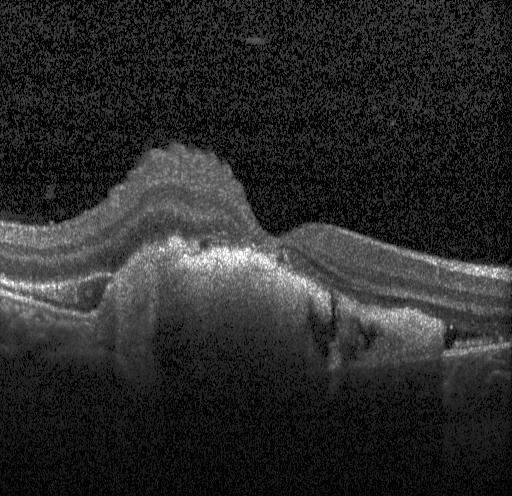 Retinal OCT cross-section; centered on the fovea; spectral-domain OCT; acquired on a Heidelberg Spectralis
Macular OCT: choroidal neovascularization.